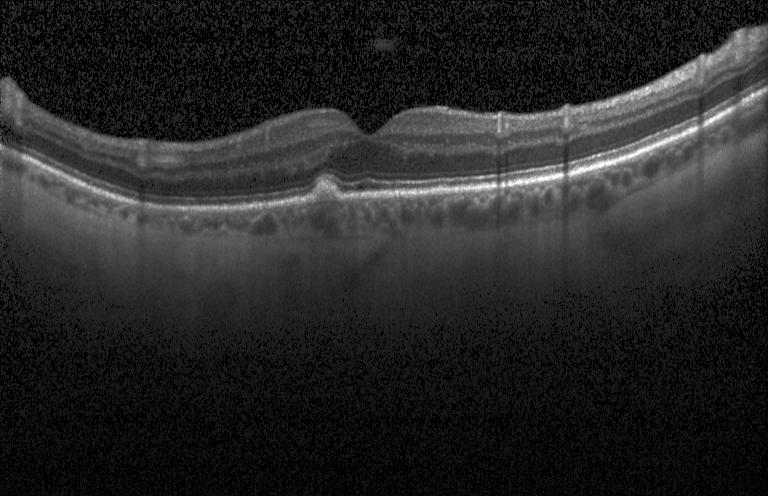

Heidelberg Spectralis OCT system; spectral-domain optical coherence tomography; optical coherence tomography scan; horizontal scan through the fovea. Macular OCT: drusen.